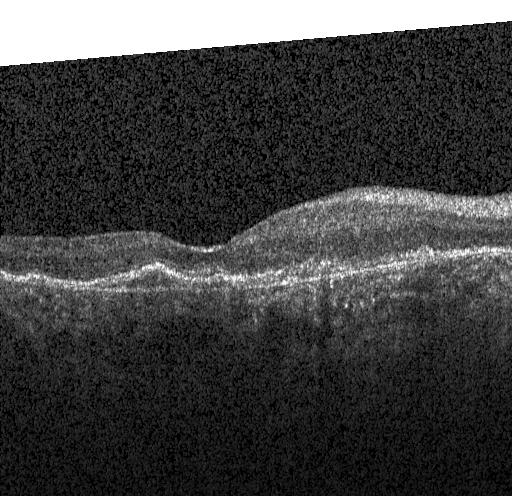

OCT scan showing a choroidal neovascular membrane.